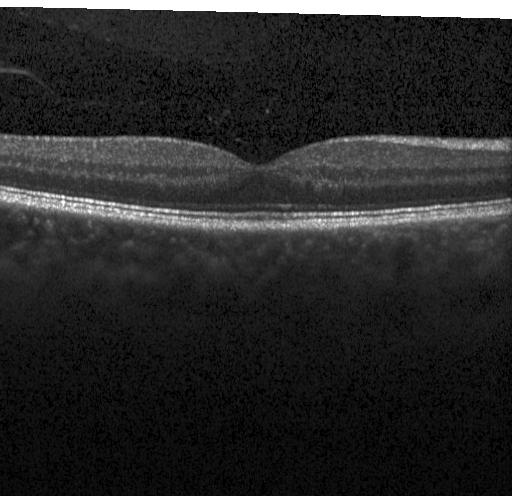 Optical coherence tomography B-scan; SD-OCT; acquired on a Heidelberg Spectralis
Dx: no evidence of CNV, DME, or drusen.